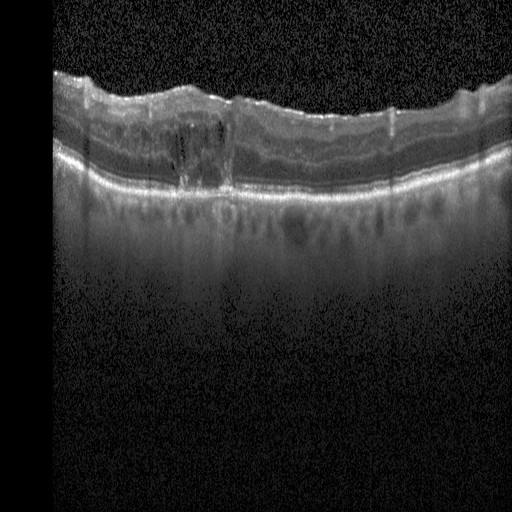
Spectral-domain OCT · instrument: Heidelberg Spectralis · horizontal scan through the fovea · OCT B-scan. Macular OCT: diabetic macular edema.